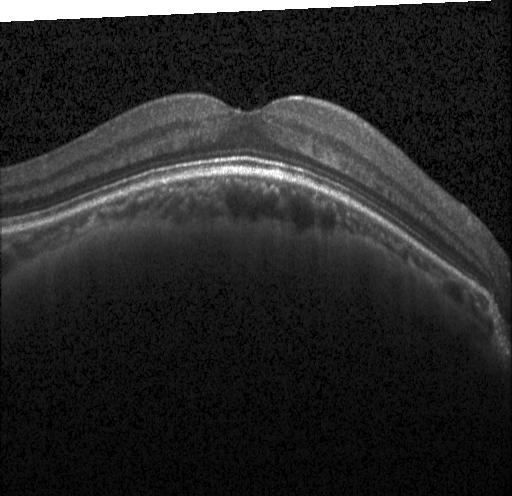

Diagnosis: no evidence of CNV, DME, or drusen.